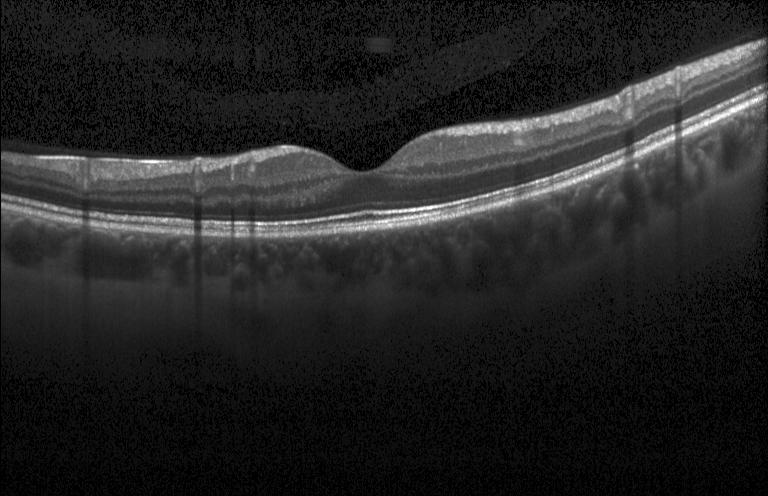
Acquired on a Heidelberg Spectralis · fovea-centered · SD-OCT · optical coherence tomography B-scan
Diagnosis: neither choroidal neovascularization, diabetic macular edema, nor drusen.